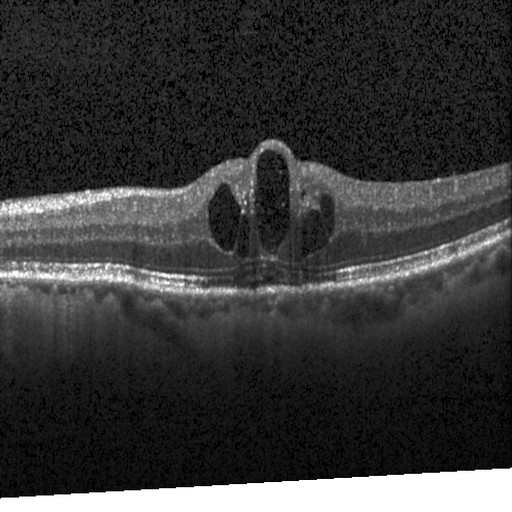
Retinal OCT B-scan. Impression: diabetic macular edema (DME).